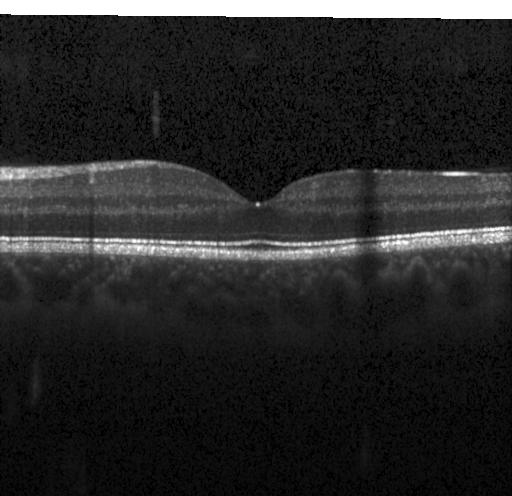
OCT scan showing neither choroidal neovascularization, diabetic macular edema, nor drusen.